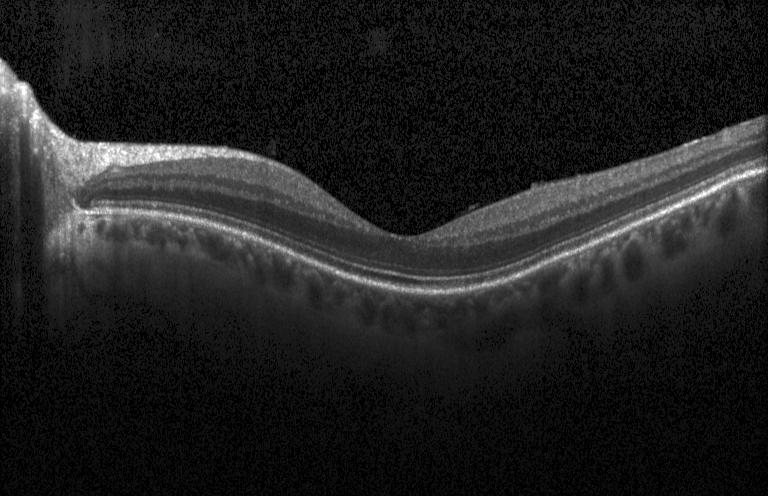

Retinal OCT cross-section. No choroidal neovascularization, no diabetic macular edema, and no drusen.